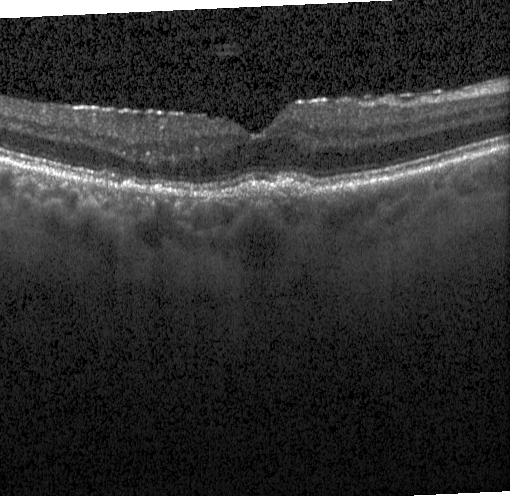

Horizontal scan through the fovea; spectral-domain OCT; OCT B-scan; Heidelberg Spectralis OCT system.
Choroidal neovascularization (CNV).